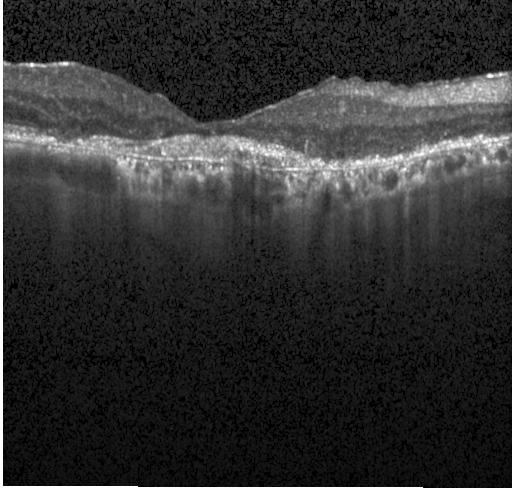

Spectral-domain OCT B-scan: a choroidal neovascular membrane.